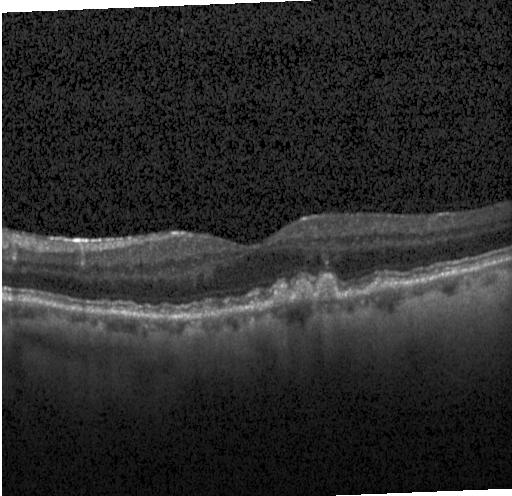

Optical coherence tomography B-scan · macular scan
Dx: drusen.